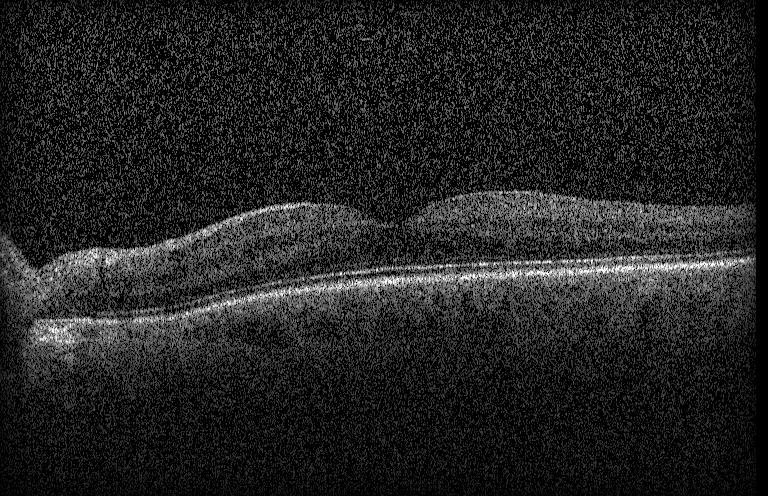

Optical coherence tomography scan
This B-scan demonstrates no choroidal neovascularization, diabetic macular edema, or drusen.